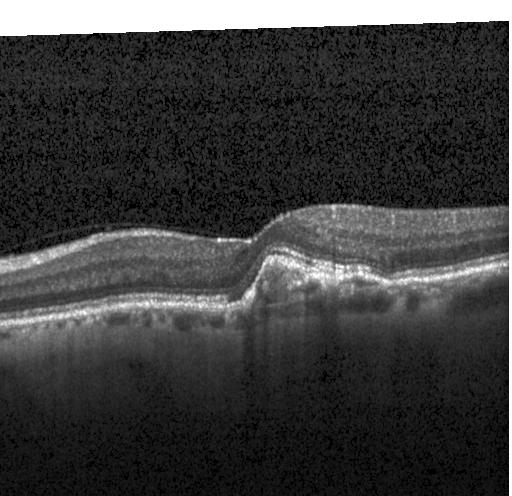 OCT finding: a choroidal neovascular membrane.